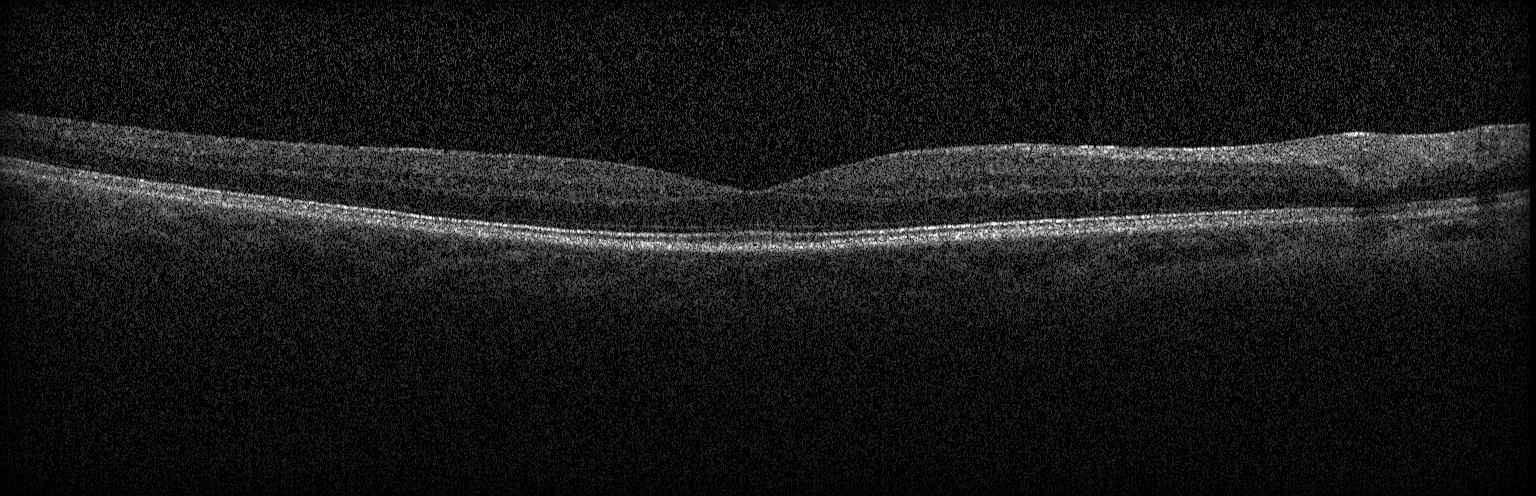 Centered on the fovea; retinal OCT cross-section; Heidelberg Spectralis OCT system; spectral-domain OCT — This B-scan demonstrates no CNV, no DME, and no drusen.